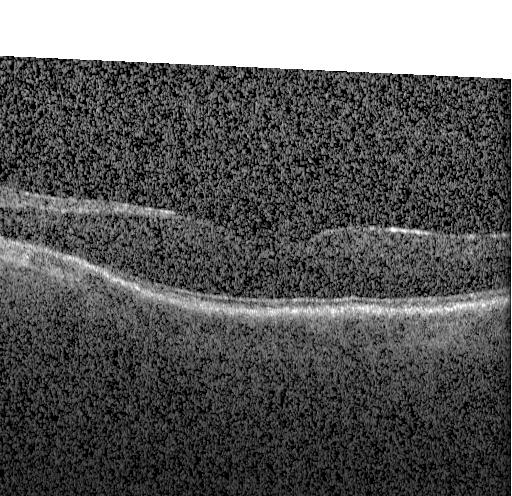

Retinal OCT B-scan, Heidelberg Spectralis OCT system.
No choroidal neovascularization, diabetic macular edema, or drusen.